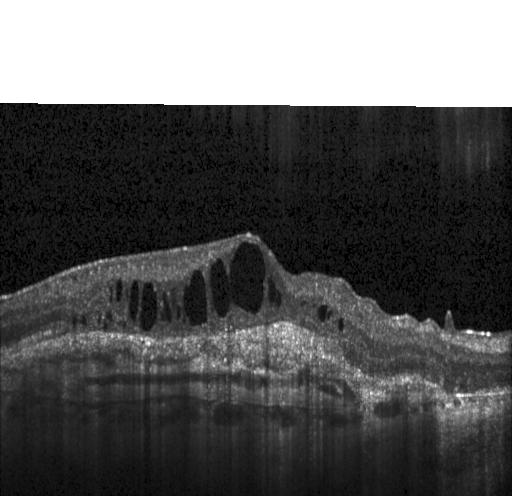

OCT B-scan — Dx: a choroidal neovascular membrane.